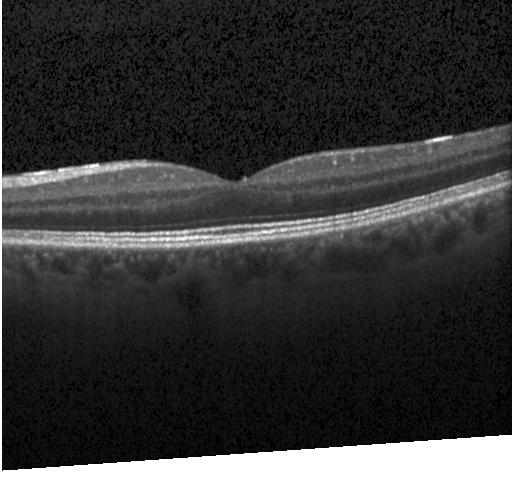 The scan shows neither CNV, DME, nor drusen.